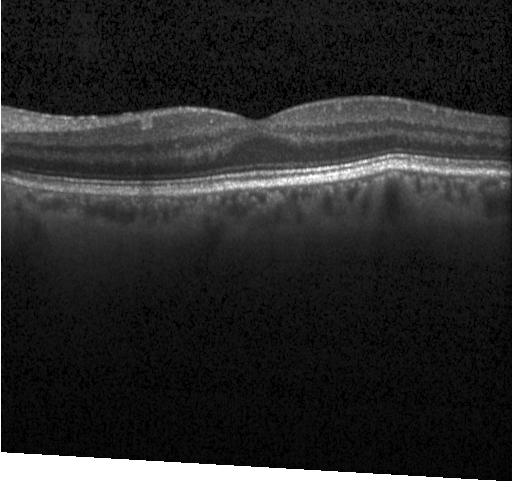

Optical coherence tomography scan. Horizontal scan through the fovea. Spectral-domain optical coherence tomography. Acquired on a Heidelberg Spectralis — Assessment: no choroidal neovascularization, no diabetic macular edema, and no drusen.